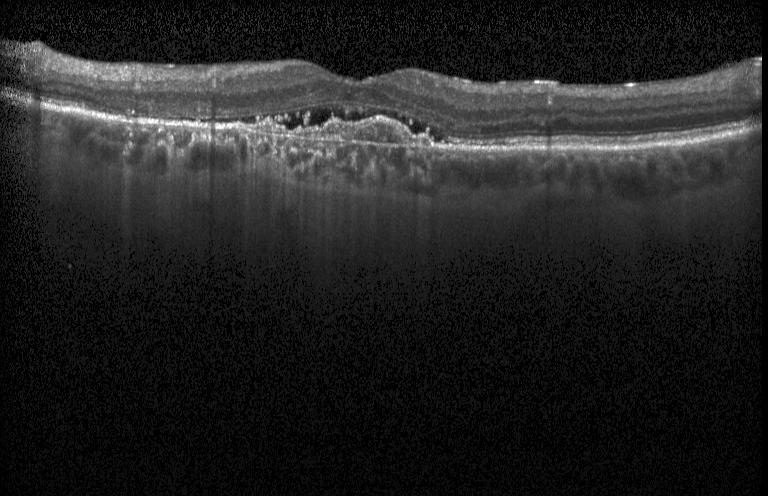 SD-OCT, retinal OCT B-scan. This B-scan demonstrates a choroidal neovascular membrane.